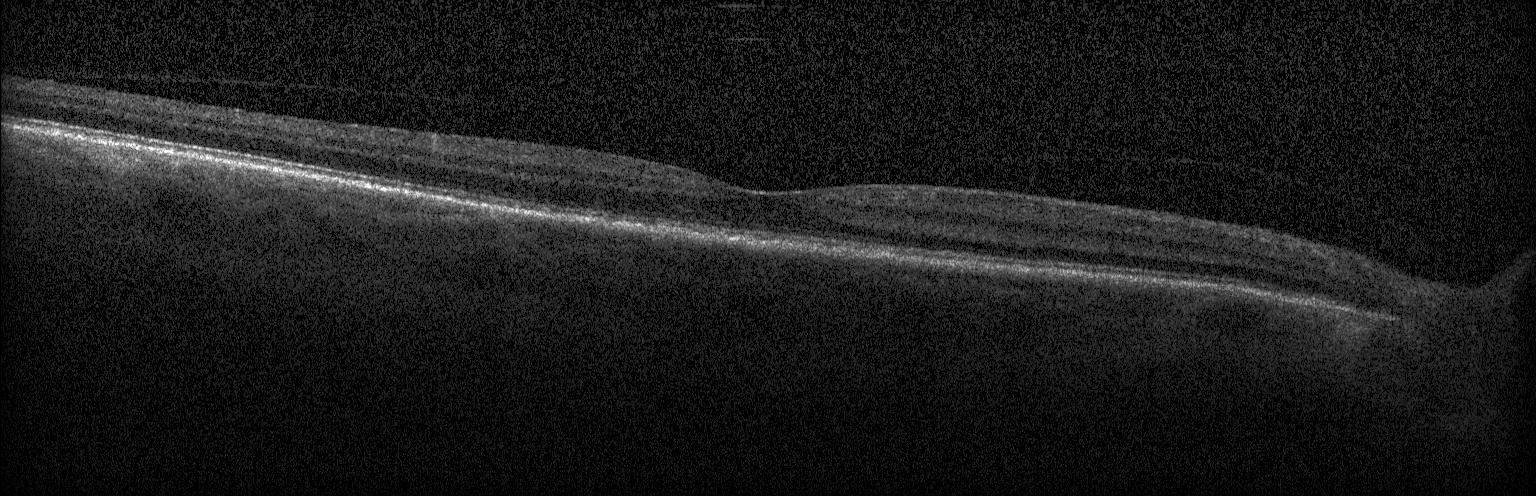 OCT B-scan. Spectral-domain optical coherence tomography. Acquired on a Heidelberg Spectralis. Centered on the fovea. Diagnosis: neither choroidal neovascularization, diabetic macular edema, nor drusen.